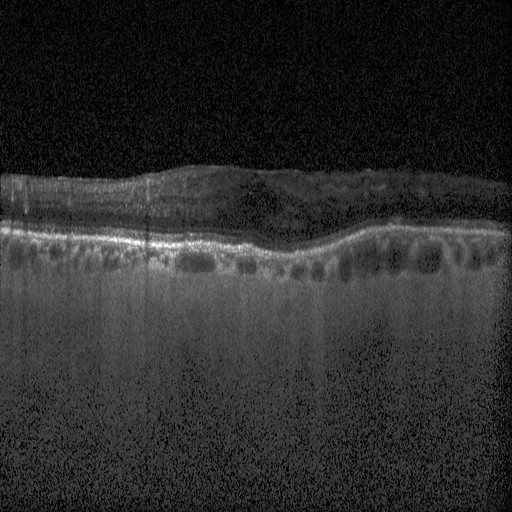

Finding: diabetic macular edema (DME).